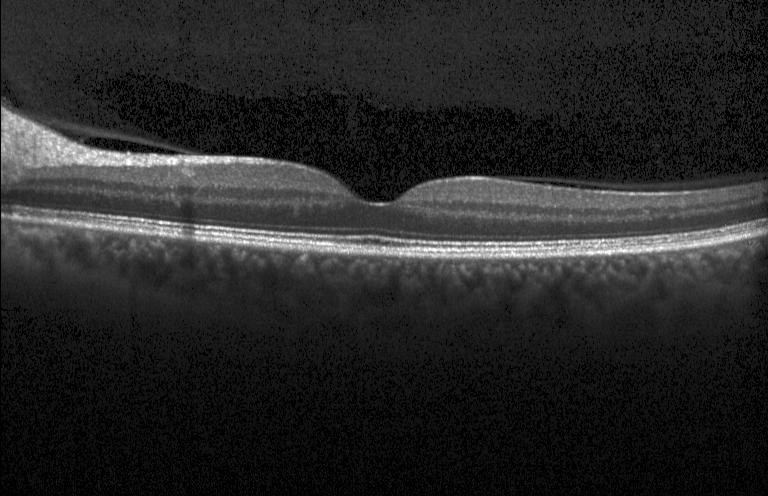 Finding: no CNV, DME, or drusen.